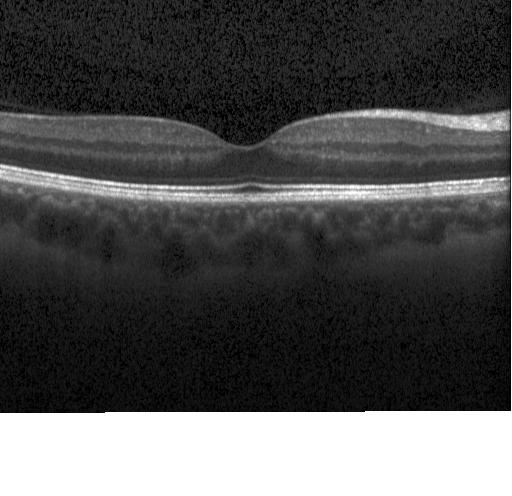
Horizontal scan through the fovea. Retinal OCT cross-section. Heidelberg Spectralis OCT system — Impression: no choroidal neovascularization, diabetic macular edema, or drusen.